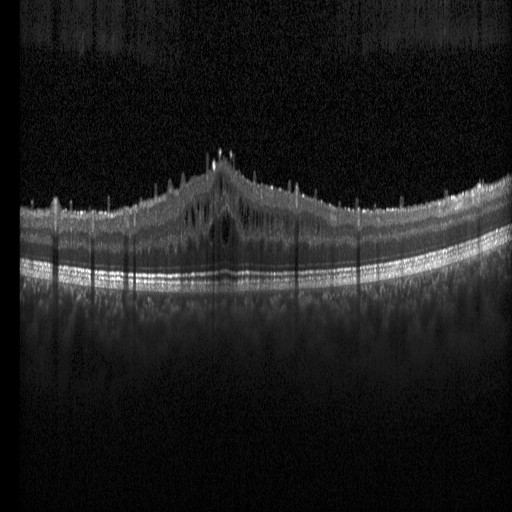

Finding: DME.